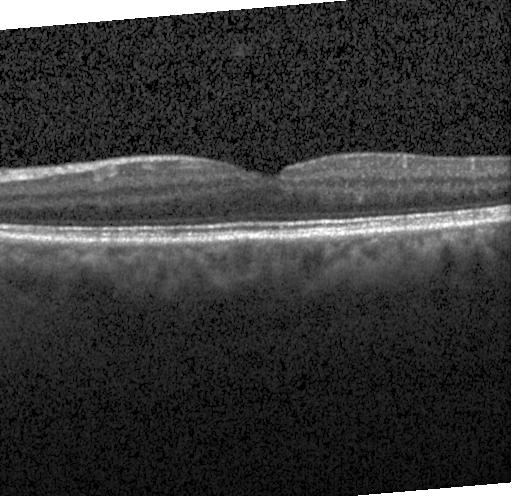
Spectral-domain optical coherence tomography · retinal OCT B-scan
Diagnosis: no choroidal neovascularization, no diabetic macular edema, and no drusen.